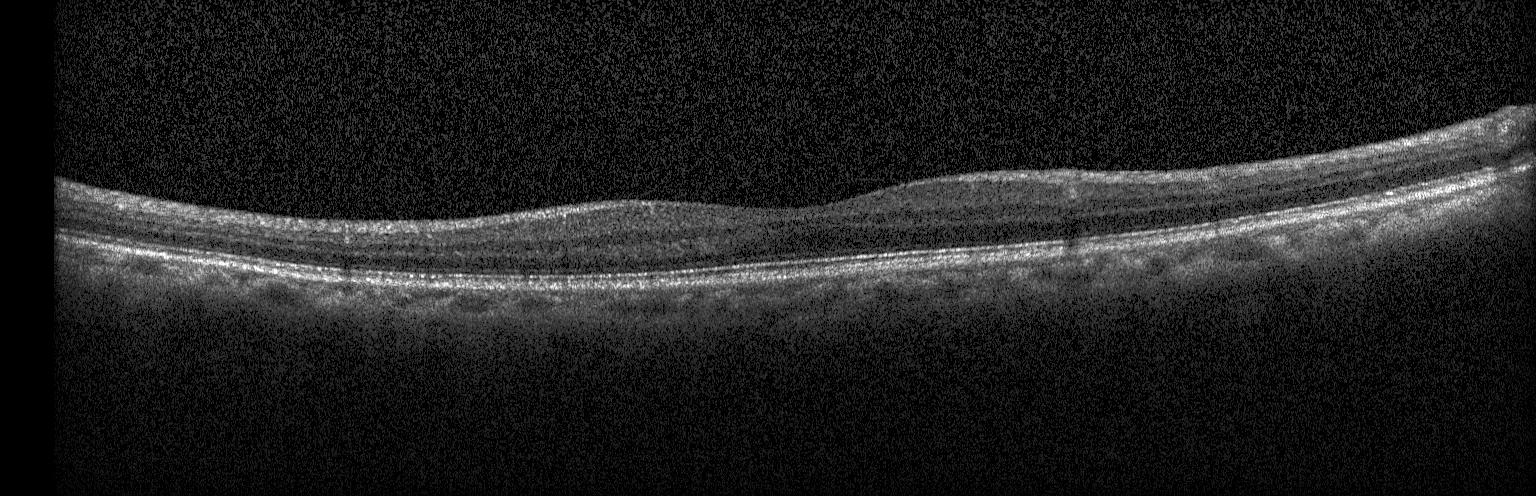

Optical coherence tomography B-scan. Spectral-domain OCT. Heidelberg Spectralis
No choroidal neovascularization, diabetic macular edema, or drusen.